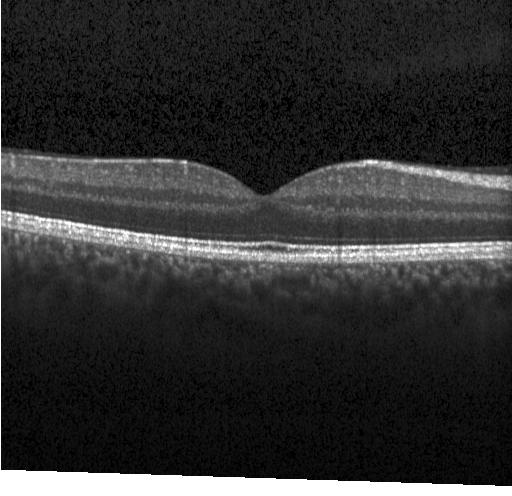 Retinal OCT cross-section showing no choroidal neovascularization, no diabetic macular edema, and no drusen.